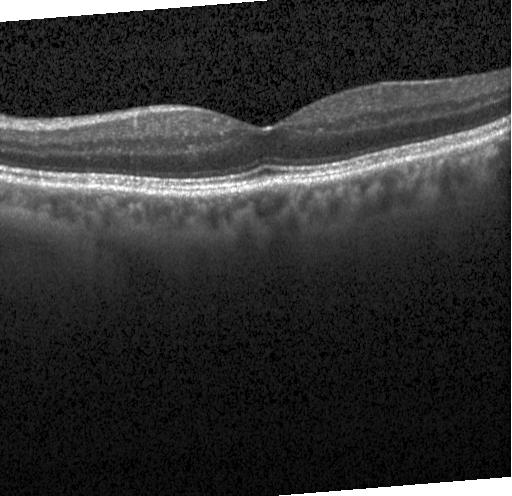

Acquired on a Heidelberg Spectralis. Spectral-domain optical coherence tomography. OCT B-scan
Finding: neither choroidal neovascularization, diabetic macular edema, nor drusen.